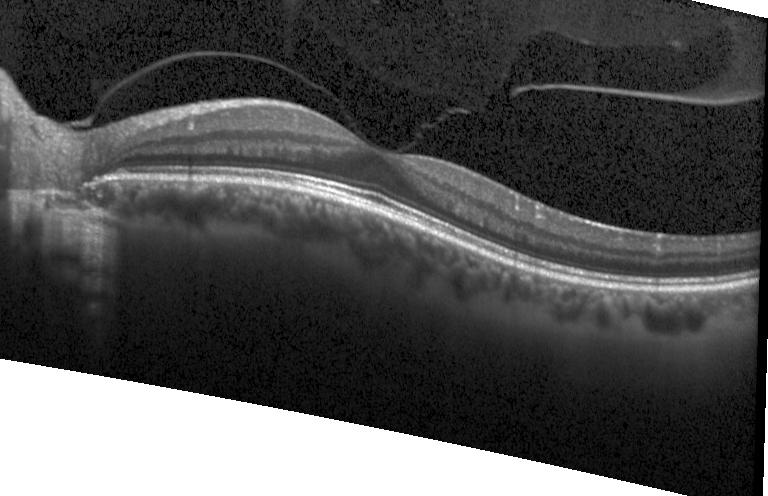
Retinal OCT cross-section, acquired on a Heidelberg Spectralis.
Macular OCT: no choroidal neovascularization, no diabetic macular edema, and no drusen.